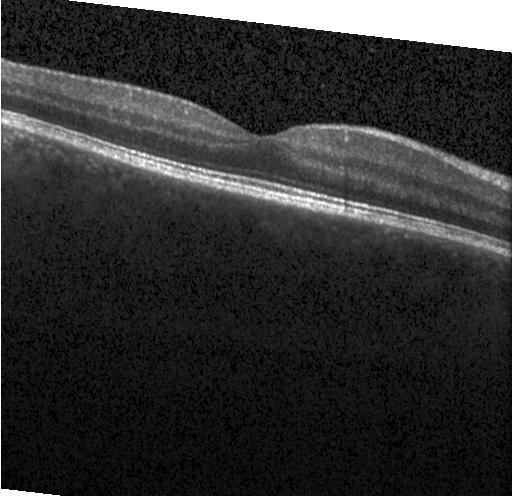 Optical coherence tomography scan.
Macular OCT: neither choroidal neovascularization, diabetic macular edema, nor drusen.